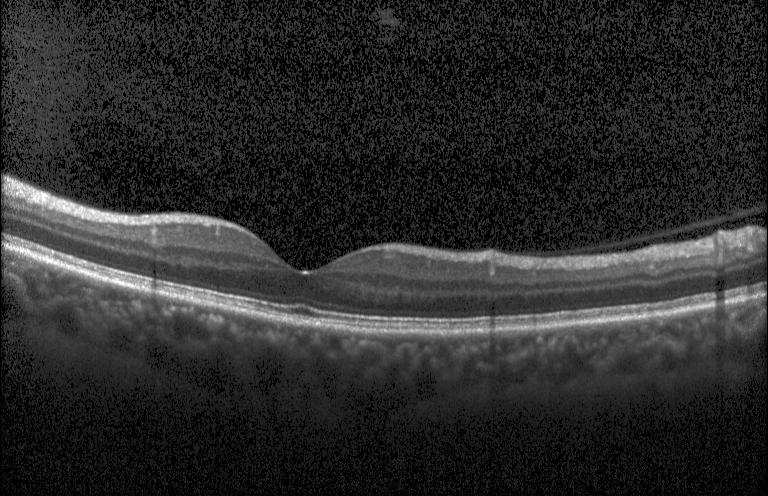
Retinal OCT cross-section showing no evidence of choroidal neovascularization, diabetic macular edema, or drusen.